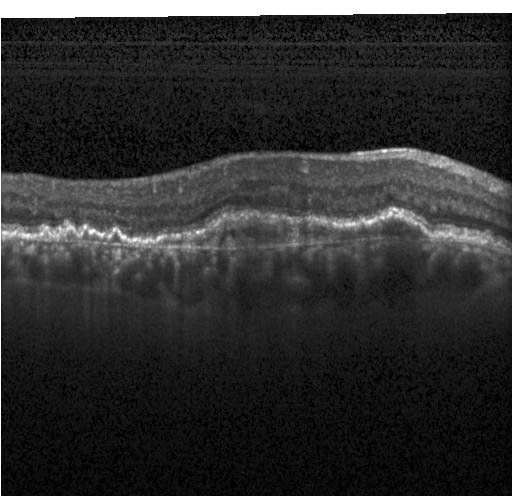 Instrument: Heidelberg Spectralis, retinal OCT cross-section
Diagnosis: CNV.